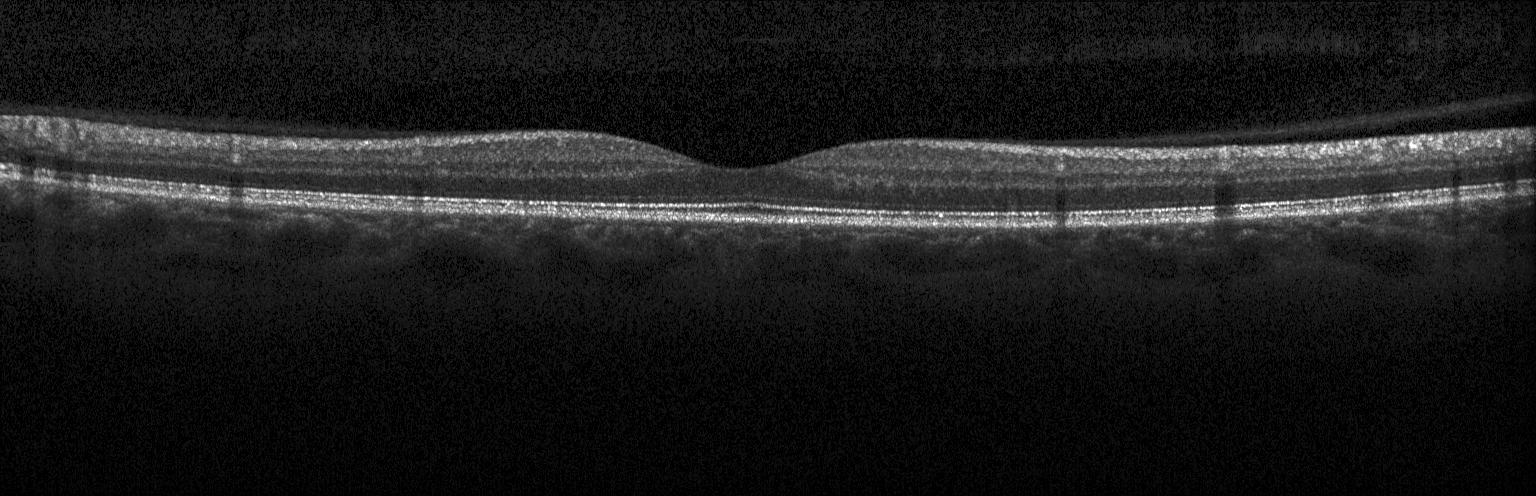

Spectral-domain OCT B-scan: no CNV, DME, or drusen.